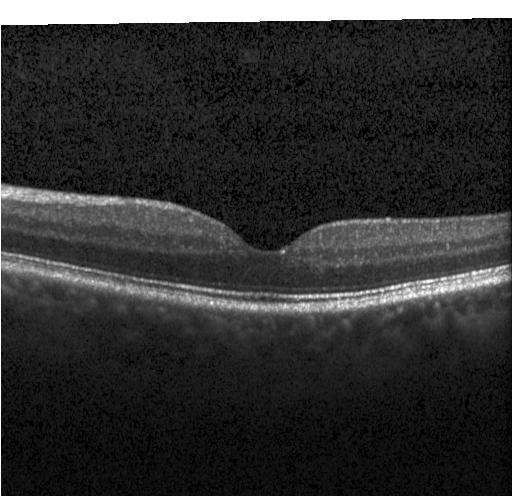

Macular OCT: no CNV, DME, or drusen.